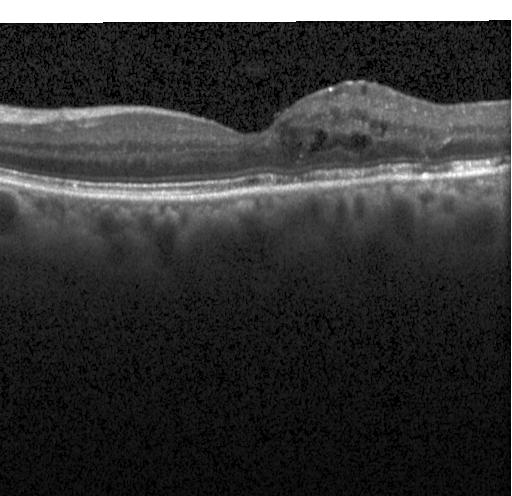
OCT B-scan; instrument: Heidelberg Spectralis; centered on the fovea
Diagnosis: diabetic macular edema.